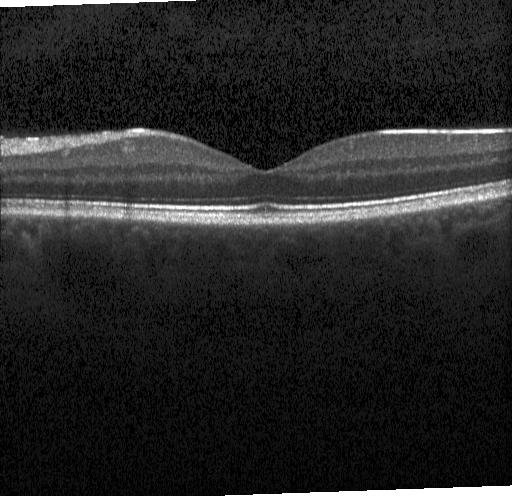

Spectral-domain optical coherence tomography; retinal OCT B-scan; instrument: Heidelberg Spectralis; fovea-centered — No choroidal neovascularization, no diabetic macular edema, and no drusen.